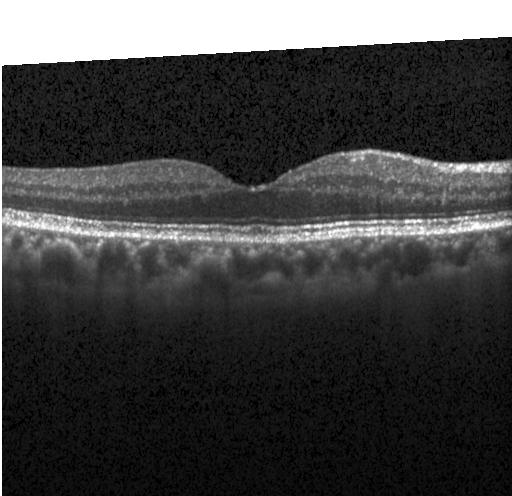

Macular scan; instrument: Heidelberg Spectralis; SD-OCT; OCT line scan. Macular OCT: no CNV, DME, or drusen.